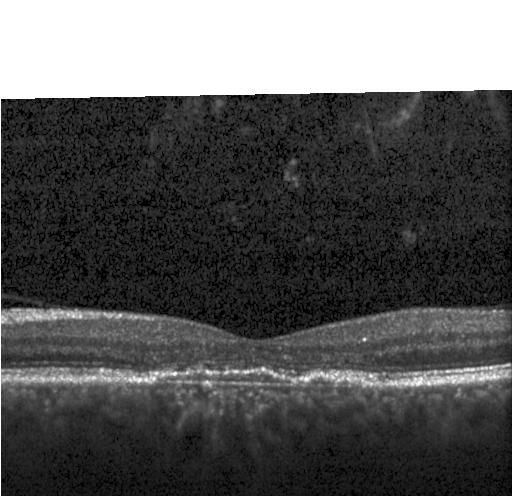 Centered on the fovea; retinal OCT cross-section
Diagnosis: choroidal neovascularization.